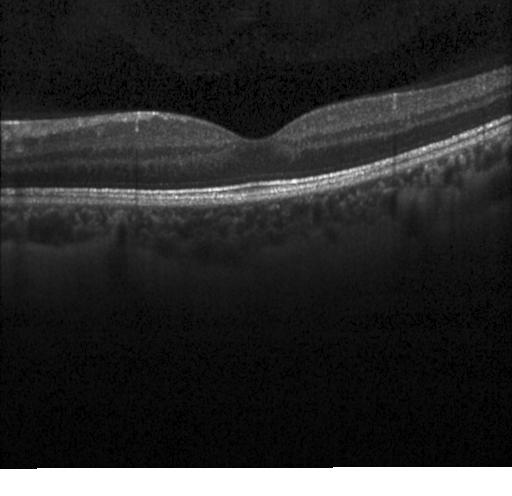
Optical coherence tomography B-scan. Through the macula.
The scan shows no evidence of CNV, DME, or drusen.